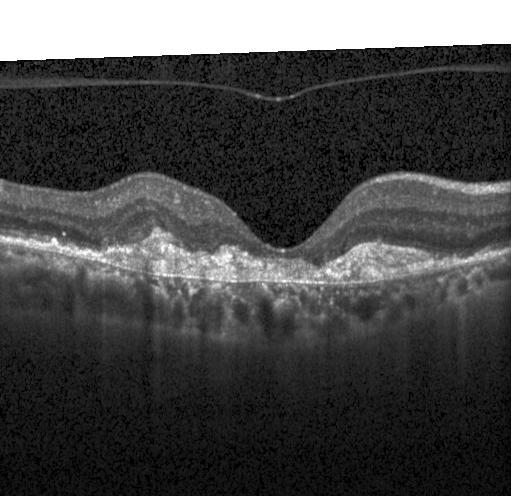

OCT B-scan.
A choroidal neovascular membrane.